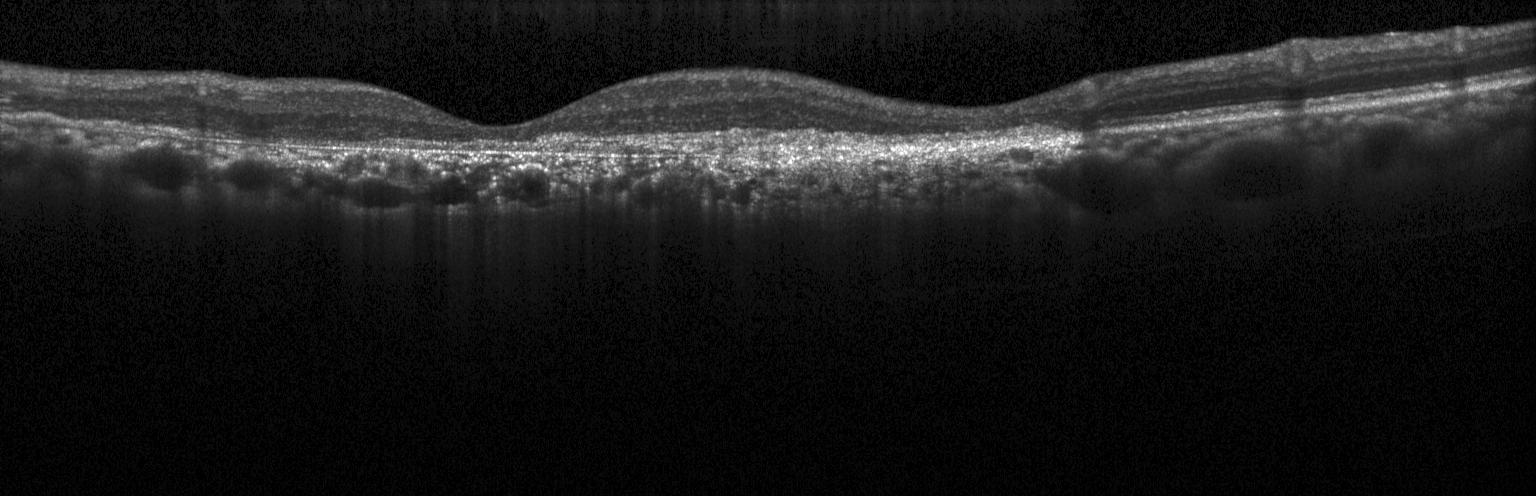

SD-OCT. Optical coherence tomography B-scan. Instrument: Heidelberg Spectralis. Fovea-centered
This B-scan demonstrates a choroidal neovascular membrane.